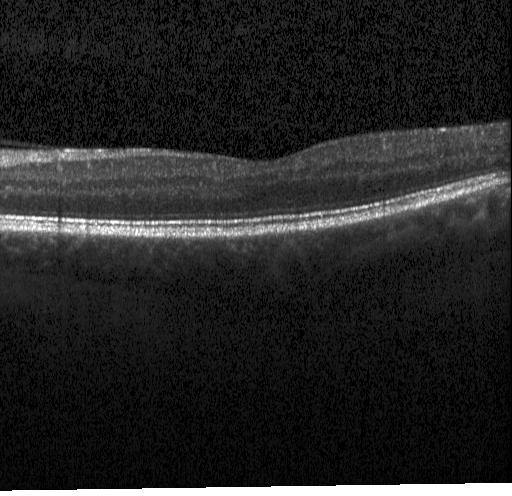

OCT B-scan — Diagnosis: no evidence of CNV, DME, or drusen.